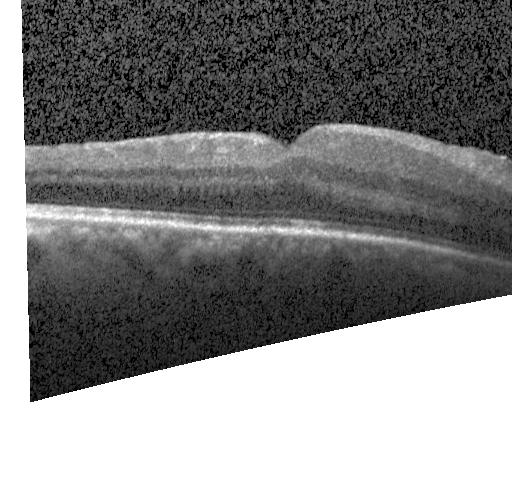
Assessment: neither choroidal neovascularization, diabetic macular edema, nor drusen.